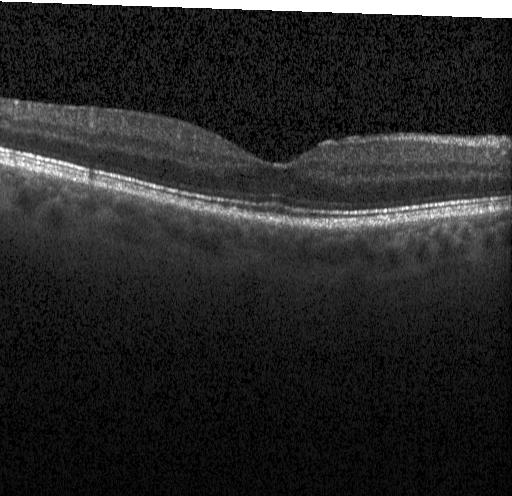 Instrument: Heidelberg Spectralis · fovea-centered · retinal OCT B-scan — This B-scan demonstrates no choroidal neovascularization, no diabetic macular edema, and no drusen.